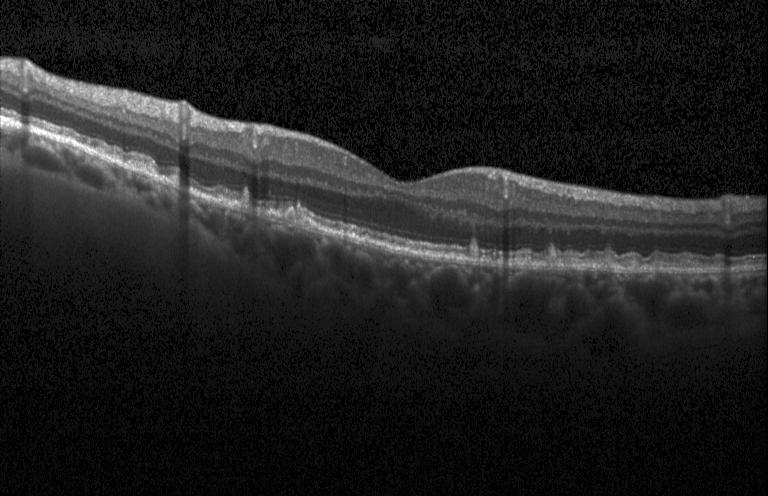
Spectral-domain OCT; optical coherence tomography B-scan
Diagnosis: sub-RPE drusenoid deposits.